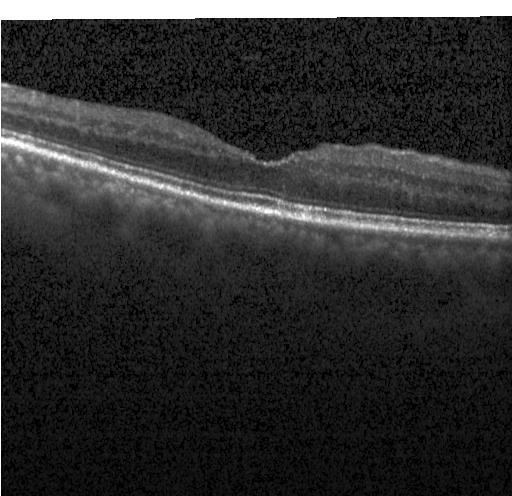

The scan shows no CNV, no DME, and no drusen.